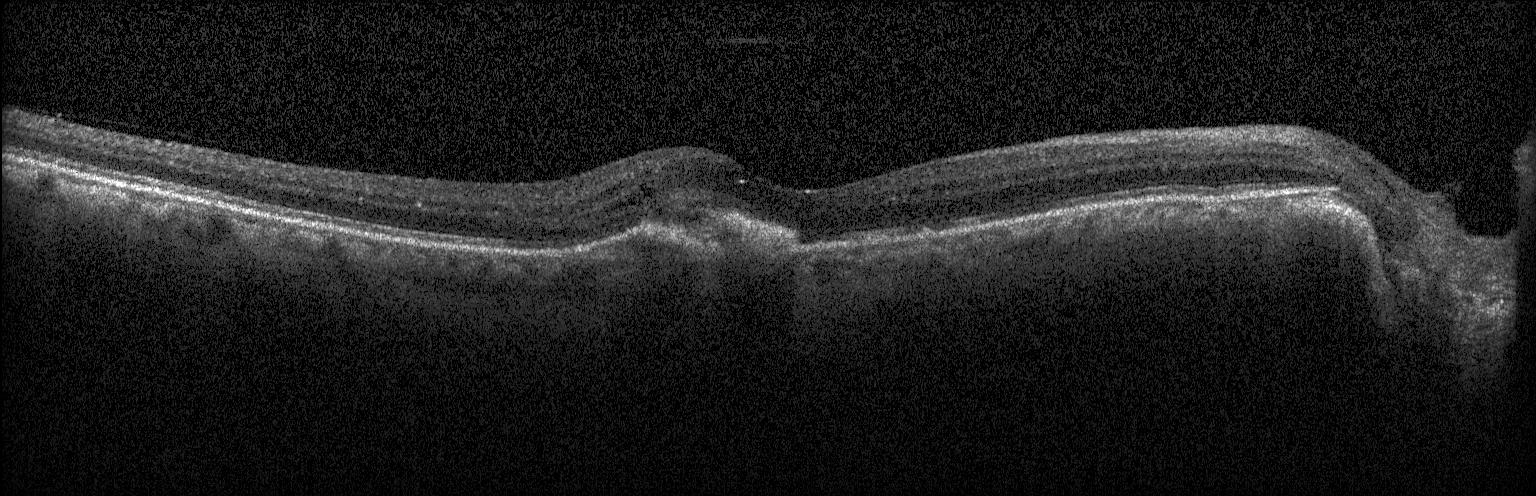

OCT B-scan showing a choroidal neovascular membrane.